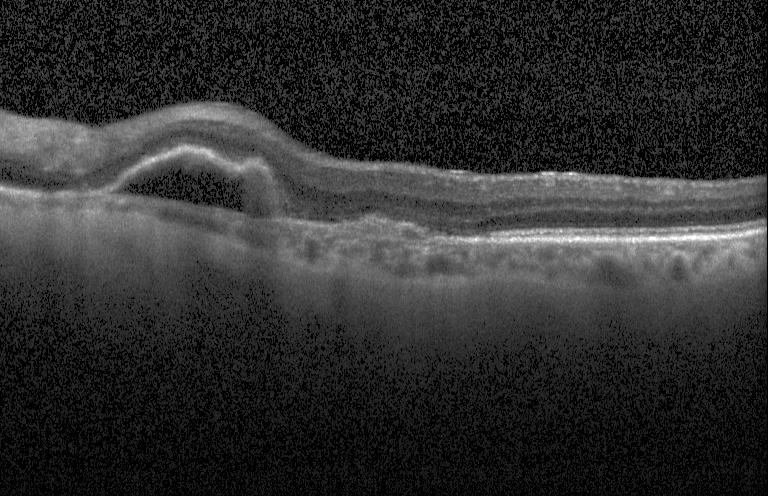

Finding: choroidal neovascularization (CNV).